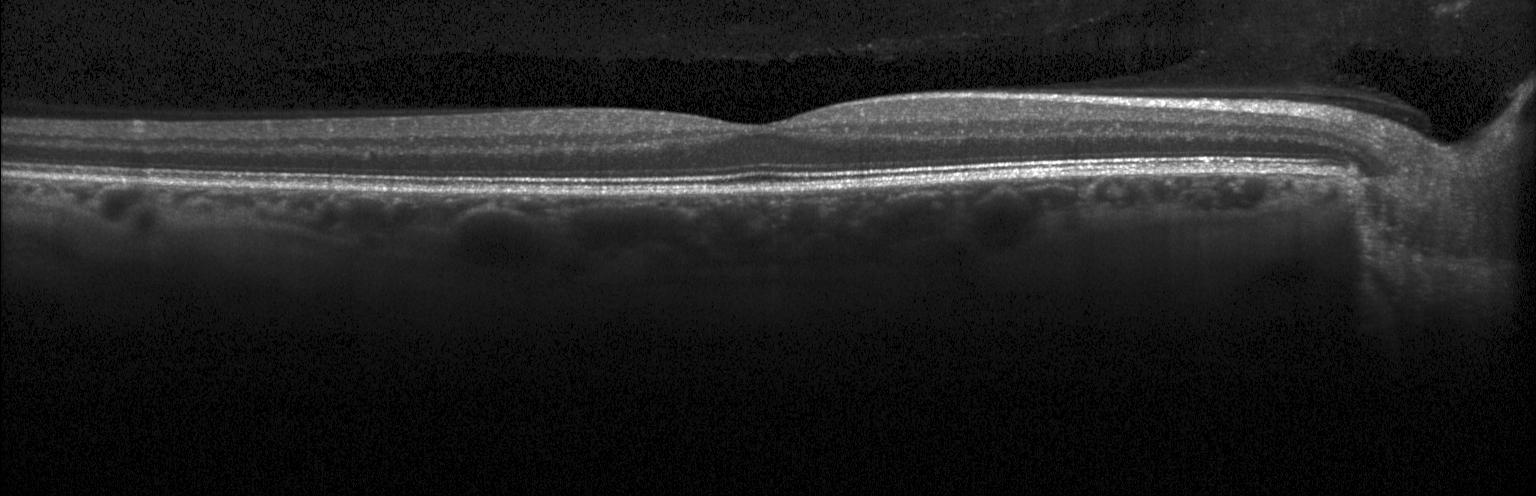

Finding: no CNV, DME, or drusen.